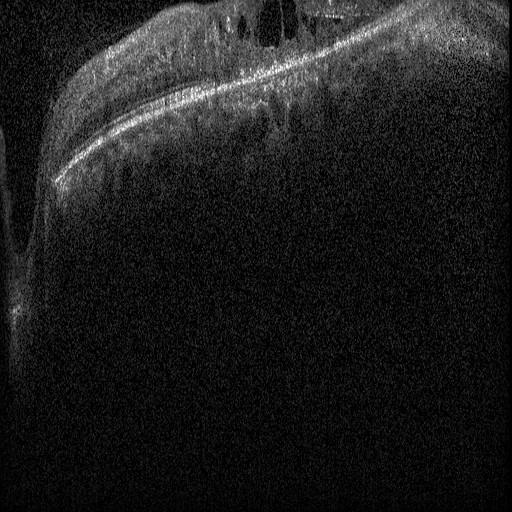 Finding: diabetic macular edema.